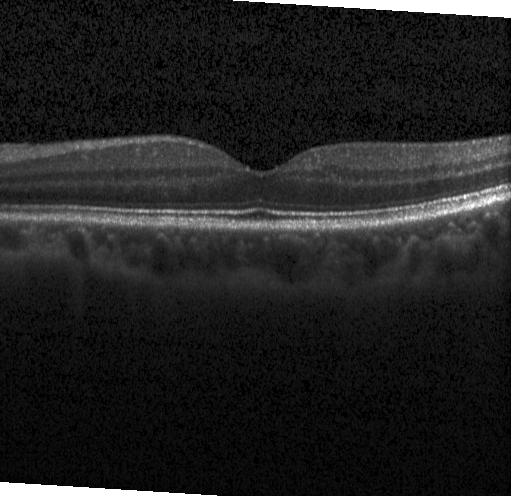
Horizontal scan through the fovea, retinal OCT cross-section — The scan shows no CNV, DME, or drusen.